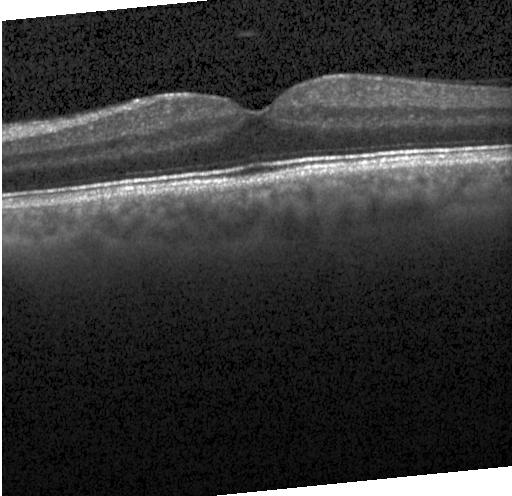
Impression: no choroidal neovascularization, no diabetic macular edema, and no drusen.